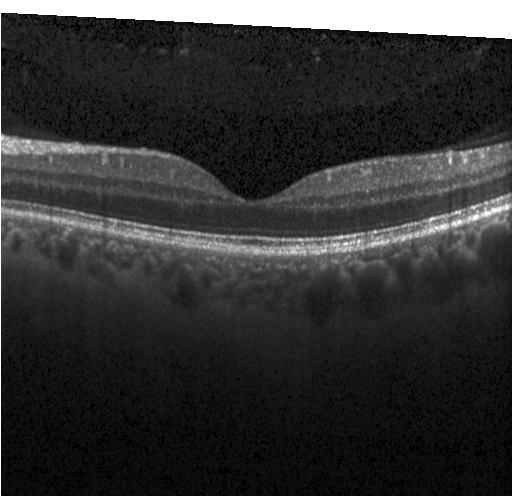
Macular OCT demonstrating neither CNV, DME, nor drusen.